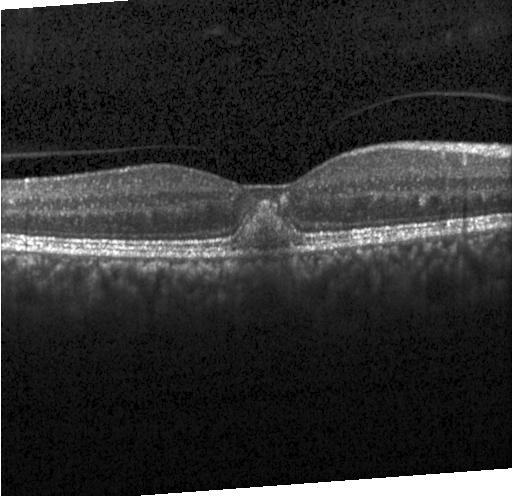 OCT B-scan
Macular OCT: a choroidal neovascular membrane.